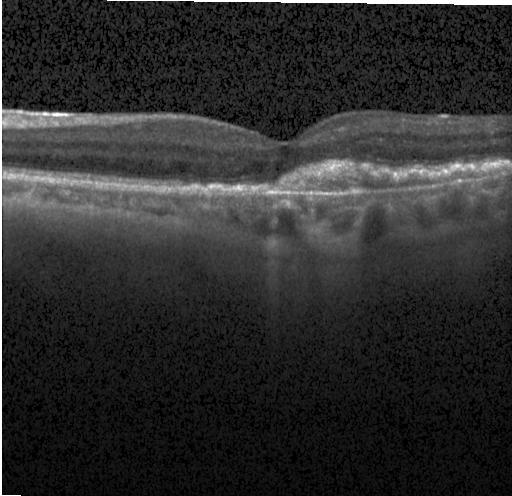
Optical coherence tomography B-scan. Macular OCT: a choroidal neovascular membrane.